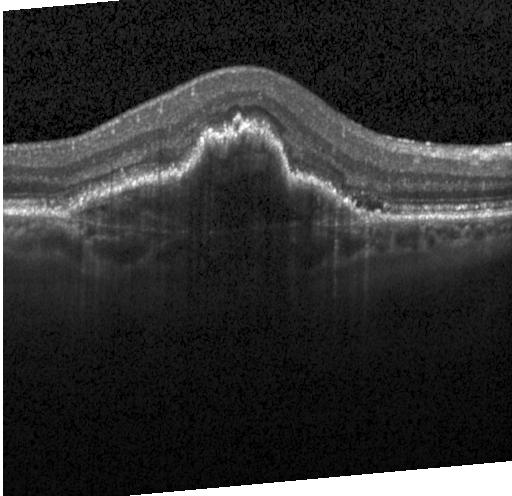
Retinal OCT B-scan; macular scan
This B-scan demonstrates a choroidal neovascular membrane.